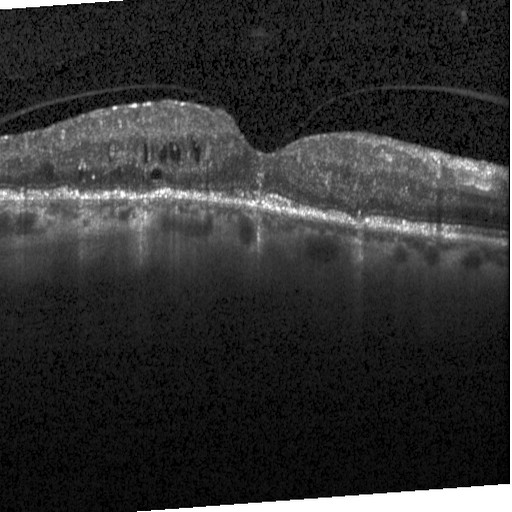 Macular OCT: DME.